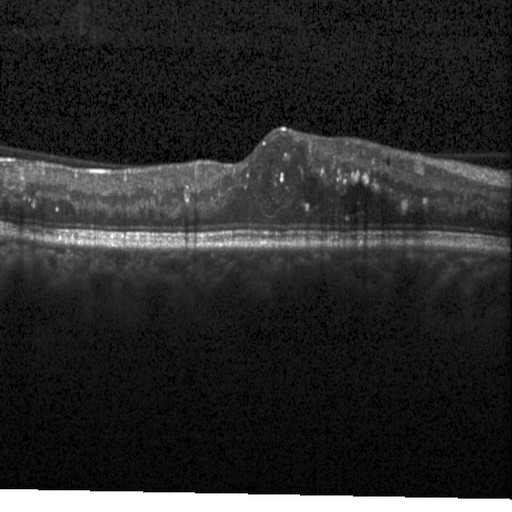
OCT line scan
Impression: diabetic macular edema (DME).